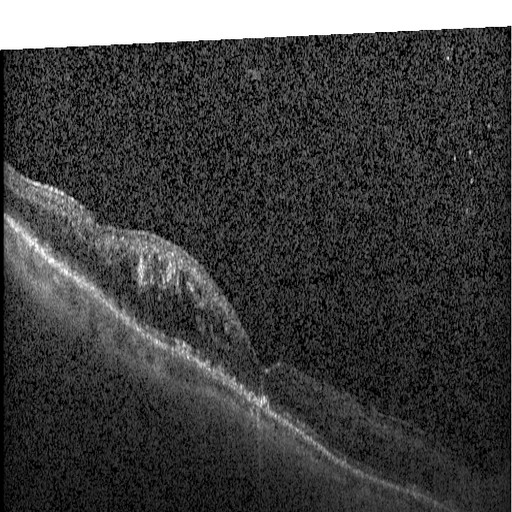

Optical coherence tomography B-scan; acquired on a Heidelberg Spectralis — Impression: diabetic macular edema (DME).